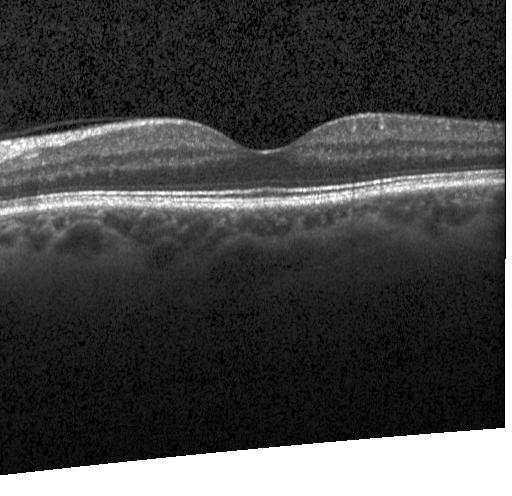 Finding: neither choroidal neovascularization, diabetic macular edema, nor drusen.